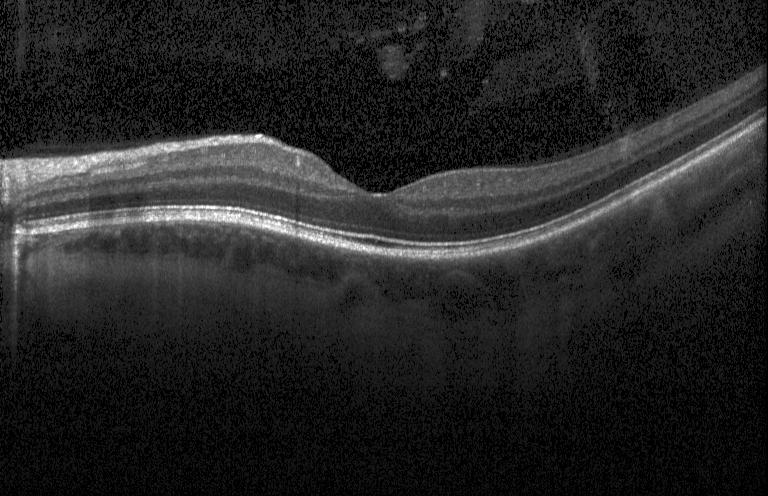

Optical coherence tomography B-scan.
Diagnosis: no choroidal neovascularization, diabetic macular edema, or drusen.